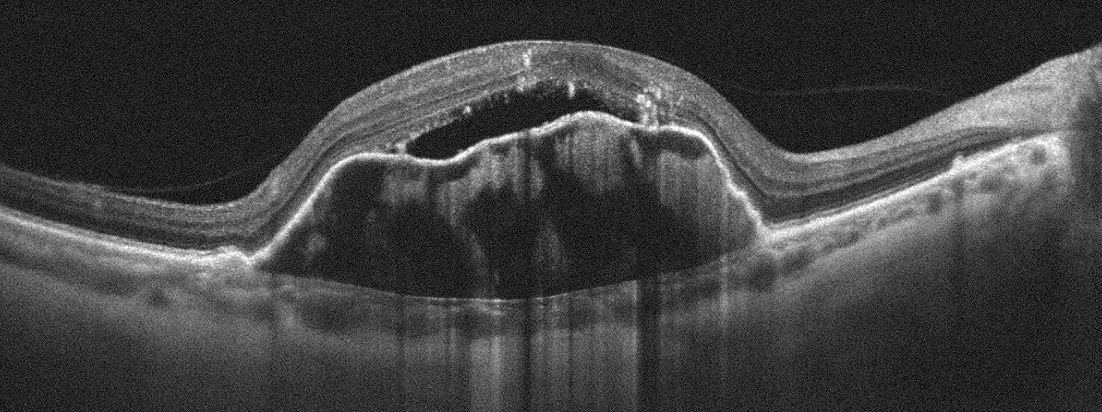 Spectral-domain OCT B-scan: age-related macular degeneration.